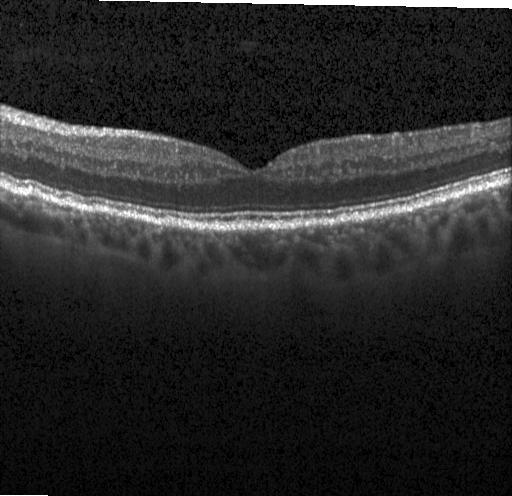 Impression: no choroidal neovascularization, no diabetic macular edema, and no drusen.